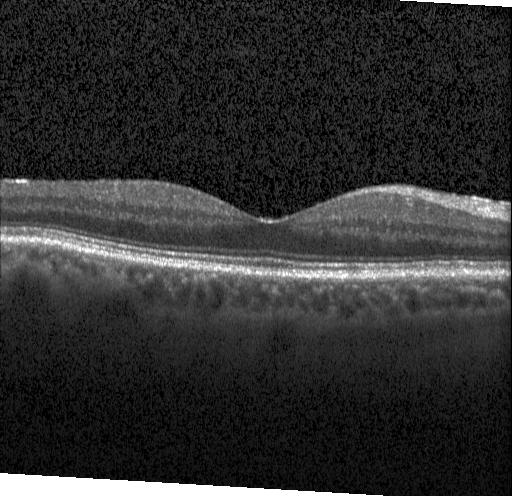
Retinal OCT B-scan
OCT finding: neither choroidal neovascularization, diabetic macular edema, nor drusen.